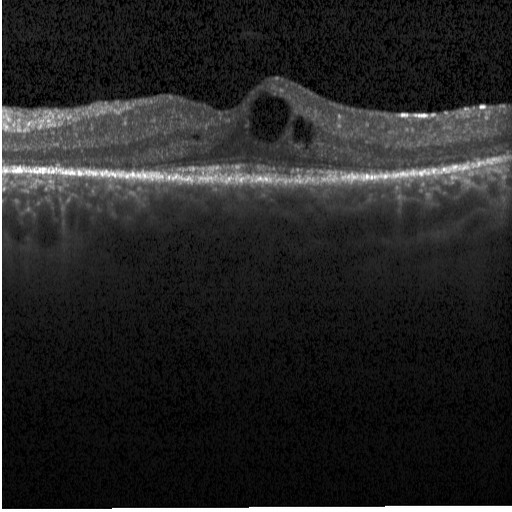 SD-OCT; optical coherence tomography B-scan; fovea-centered — Finding: diabetic macular edema.